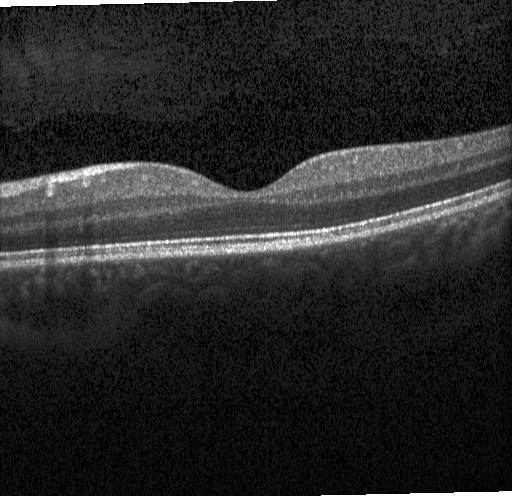

Optical coherence tomography B-scan. SD-OCT. Heidelberg Spectralis OCT system — Assessment: no choroidal neovascularization, no diabetic macular edema, and no drusen.